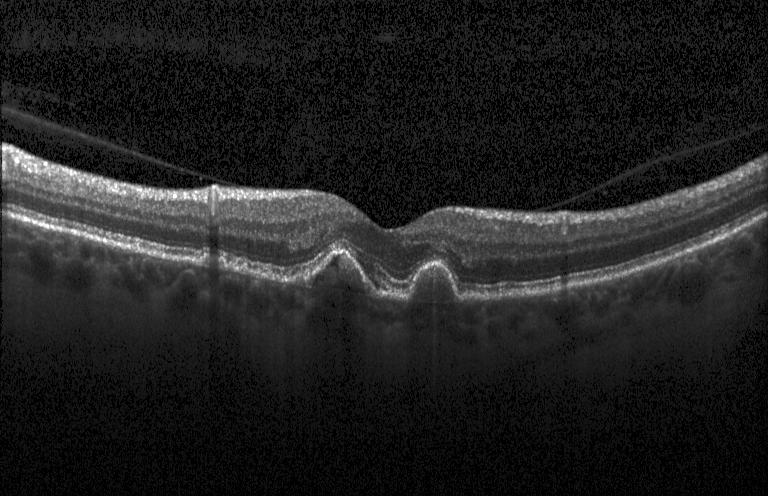

OCT B-scan, spectral-domain OCT, macular scan, acquired on a Heidelberg Spectralis. Diagnosis: sub-RPE drusenoid deposits.